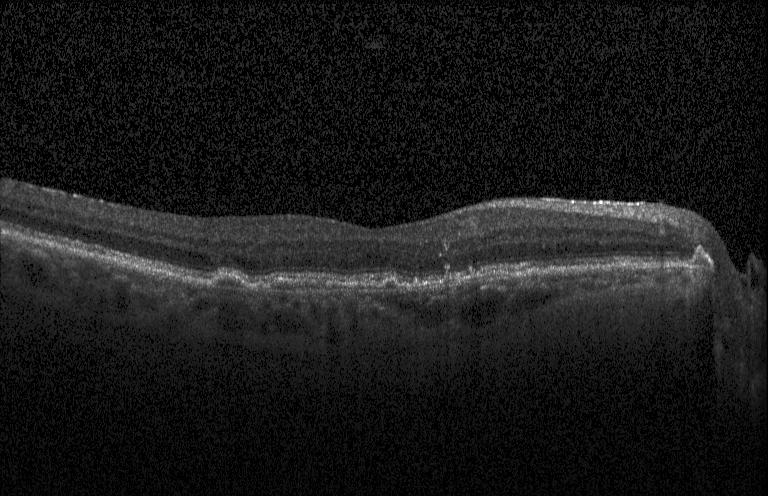 SD-OCT, through the macula, acquired on a Heidelberg Spectralis, retinal OCT cross-section. Choroidal neovascularization.